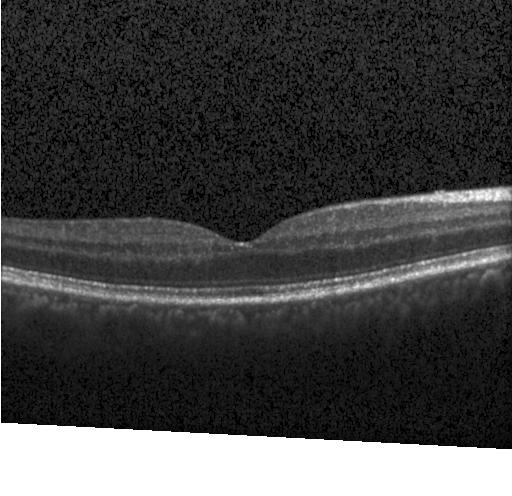
Finding: no CNV, DME, or drusen.